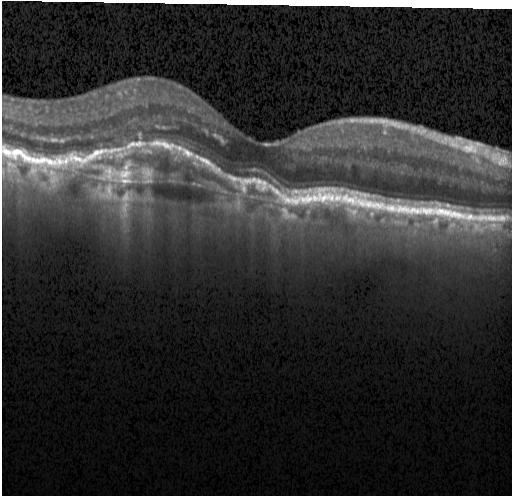
This B-scan demonstrates choroidal neovascularization (CNV).